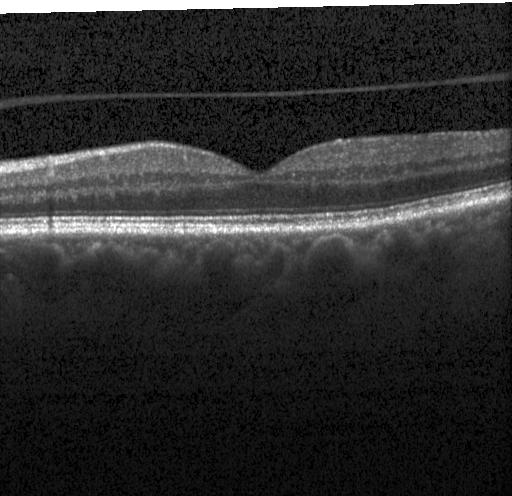

Diagnosis: no choroidal neovascularization, no diabetic macular edema, and no drusen.